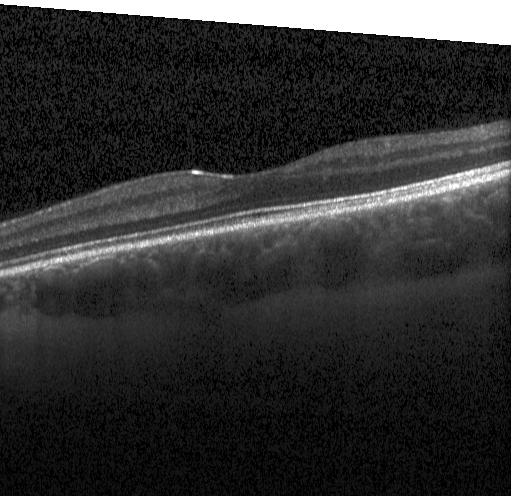 OCT B-scan — Finding: no evidence of CNV, DME, or drusen.